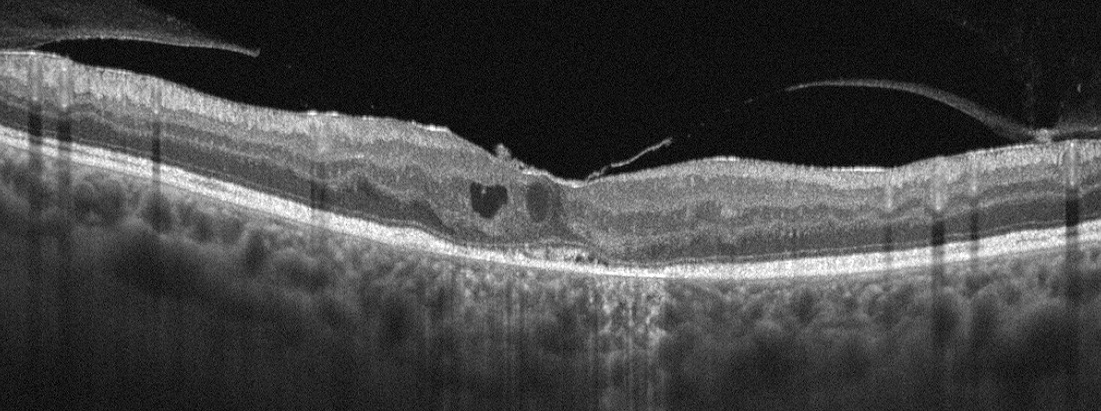
Impression: DME.